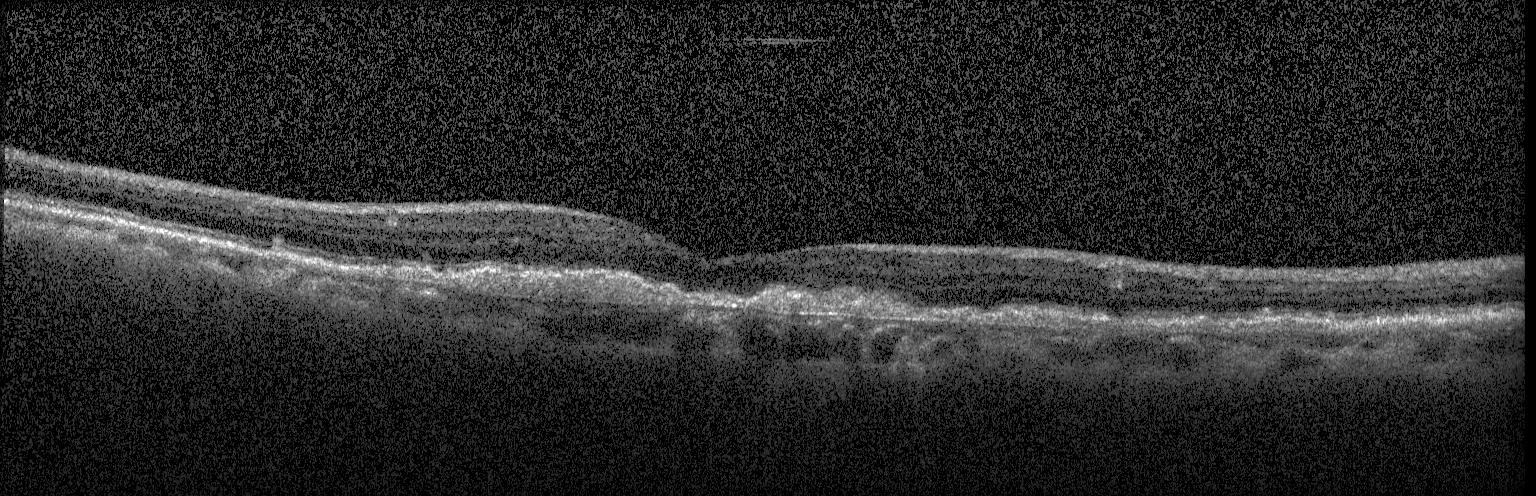 Optical coherence tomography B-scan — Assessment: choroidal neovascularization.